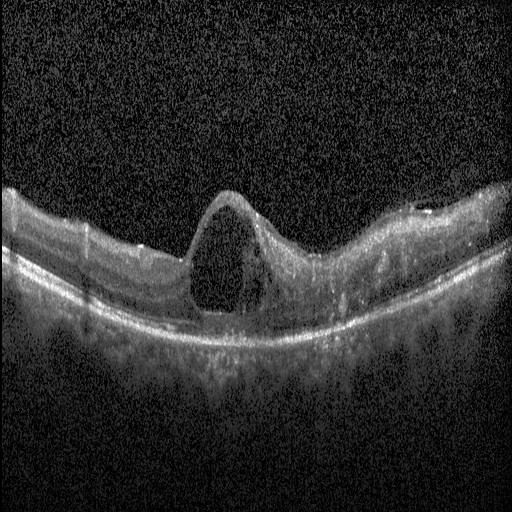

Optical coherence tomography B-scan — Impression: DME.